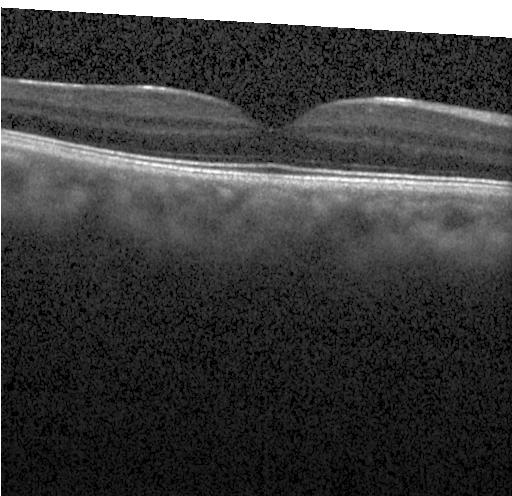
Optical coherence tomography B-scan; spectral-domain OCT; instrument: Heidelberg Spectralis; macular scan — OCT finding: no choroidal neovascularization, diabetic macular edema, or drusen.